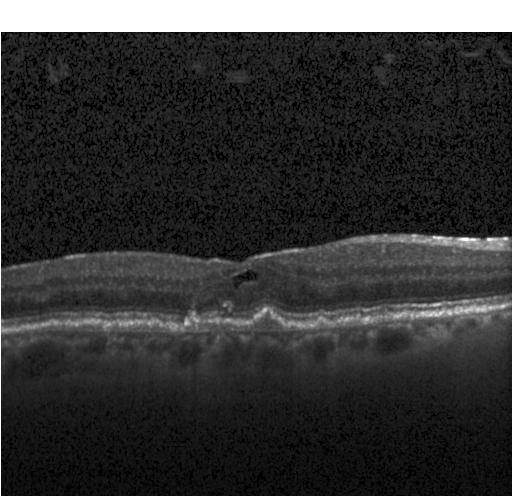

Macular scan · OCT B-scan · SD-OCT · Heidelberg Spectralis OCT system.
Diagnosis: a choroidal neovascular membrane.